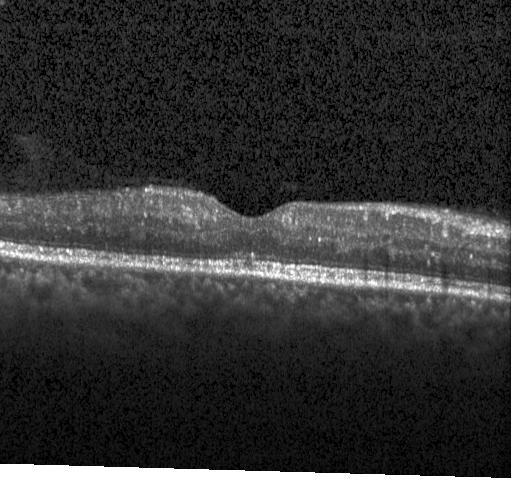

Optical coherence tomography B-scan, centered on the fovea. This B-scan demonstrates diabetic macular edema.